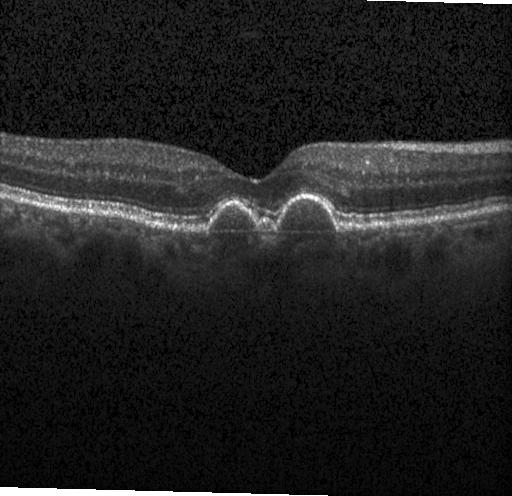 Through the macula · OCT B-scan · SD-OCT. Assessment: multiple drusen.